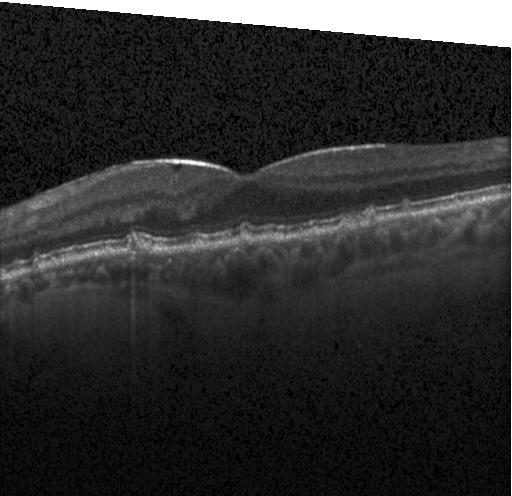
Finding: multiple drusen.